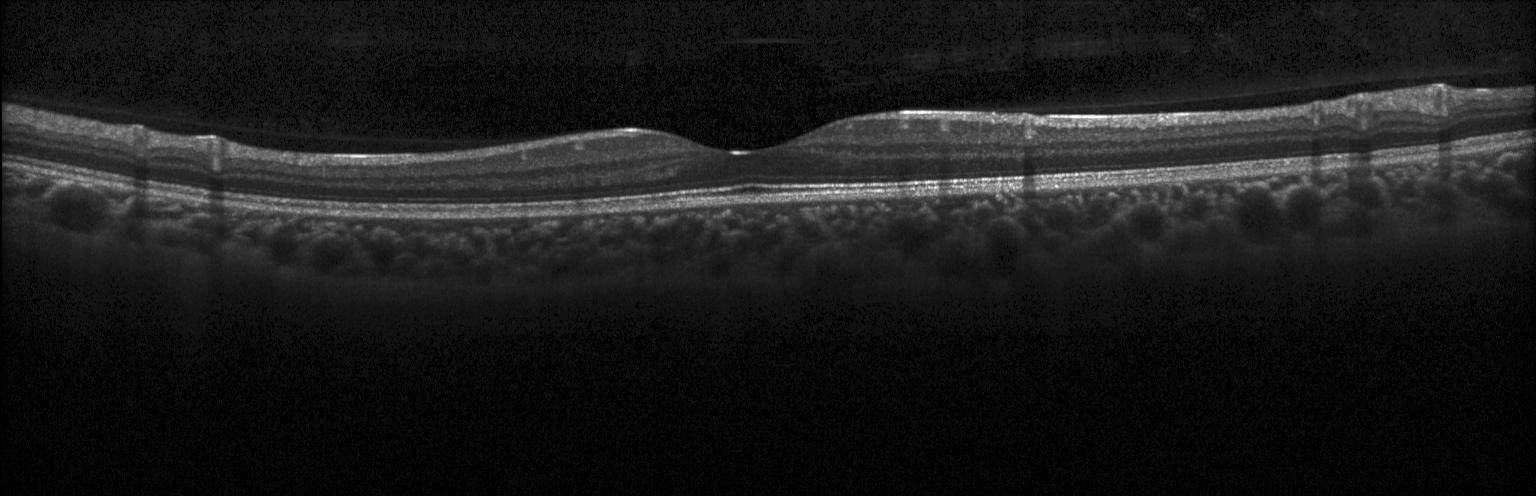

Spectral-domain OCT B-scan: no CNV, no DME, and no drusen.